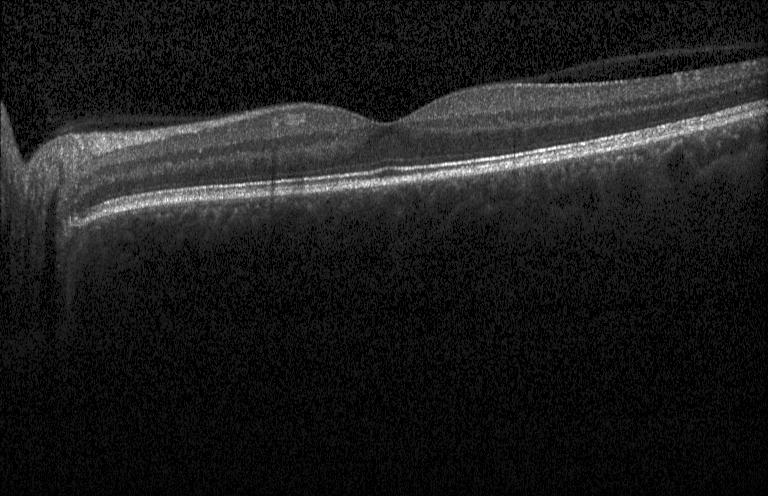 Finding: no choroidal neovascularization, diabetic macular edema, or drusen.